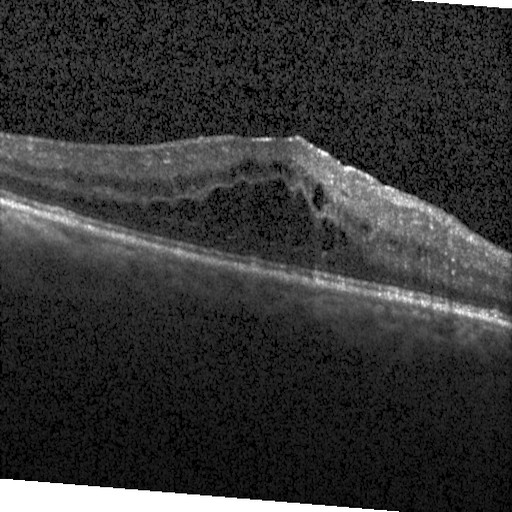 Macular OCT demonstrating DME.